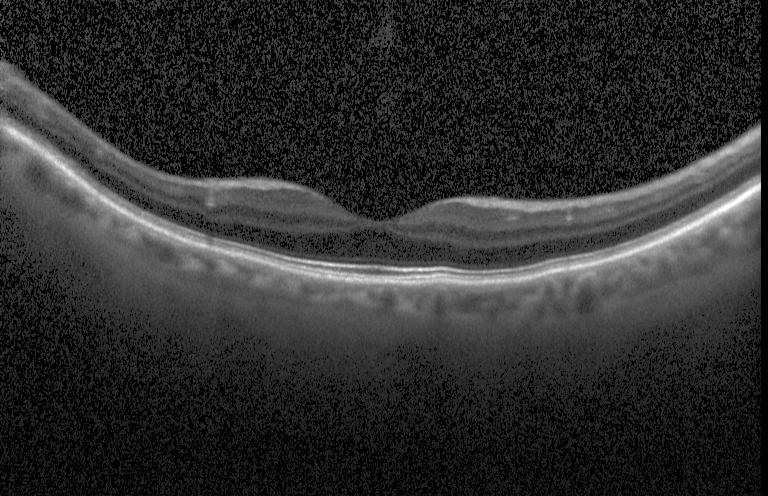 Diagnosis: no evidence of choroidal neovascularization, diabetic macular edema, or drusen.